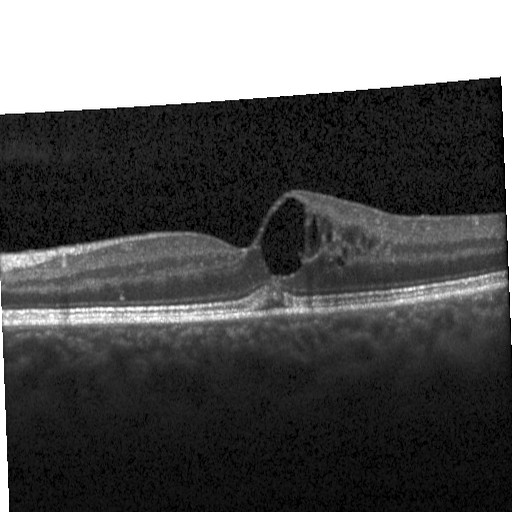 Optical coherence tomography scan. Instrument: Heidelberg Spectralis.
Diabetic macular edema.